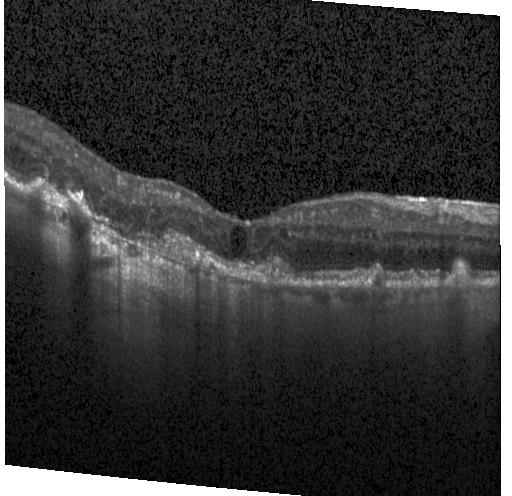
Spectral-domain optical coherence tomography. Optical coherence tomography B-scan. Horizontal scan through the fovea. Heidelberg Spectralis OCT system — Impression: CNV.